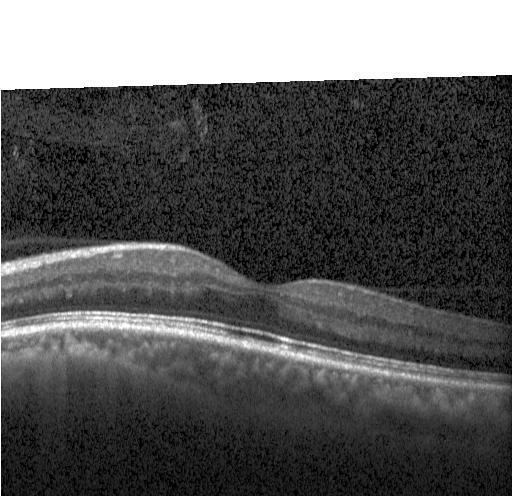

The scan shows neither choroidal neovascularization, diabetic macular edema, nor drusen.